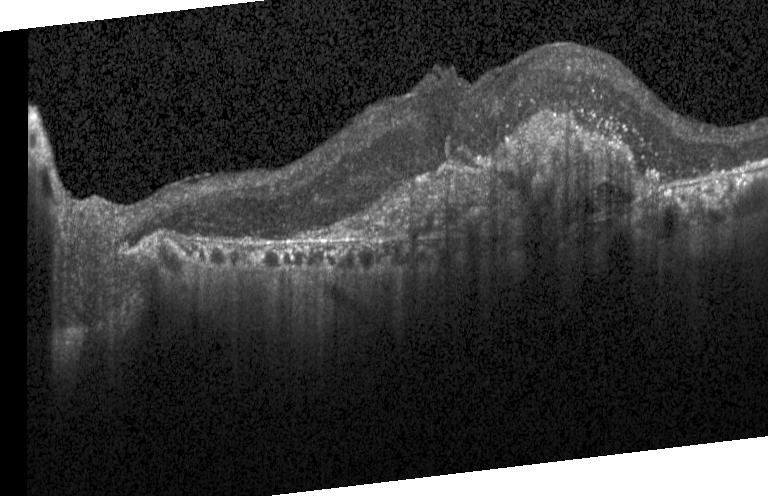 Heidelberg Spectralis · retinal OCT B-scan.
Impression: CNV.